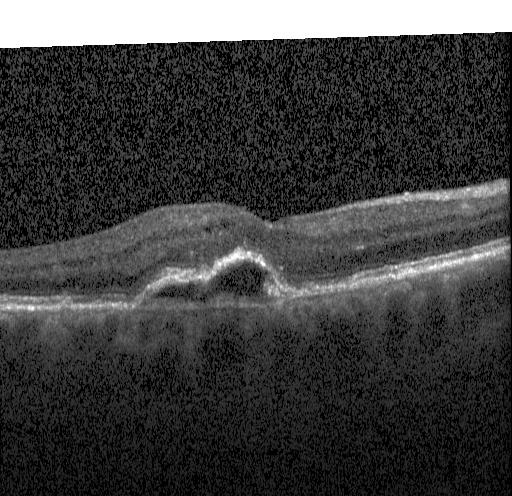 Spectral-domain OCT B-scan: a choroidal neovascular membrane.